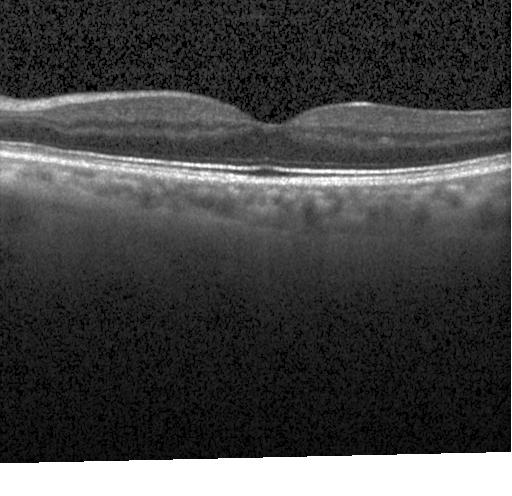 The scan shows no evidence of CNV, DME, or drusen.